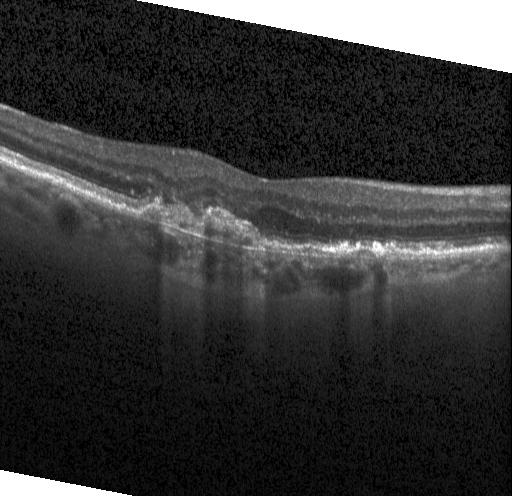

Centered on the fovea, retinal OCT B-scan.
Assessment: a choroidal neovascular membrane.